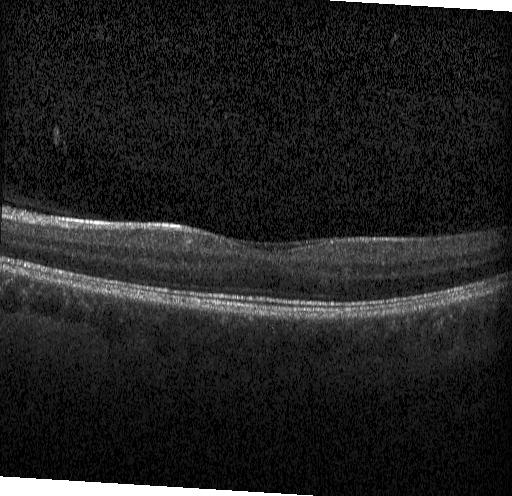
Optical coherence tomography scan, Heidelberg Spectralis OCT system. Macular OCT: no evidence of choroidal neovascularization, diabetic macular edema, or drusen.